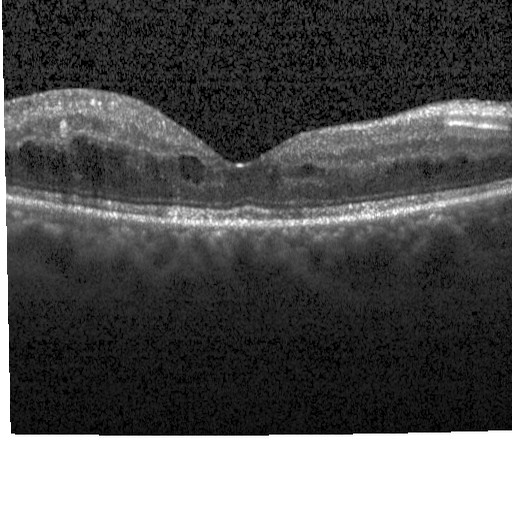
Dx: DME.